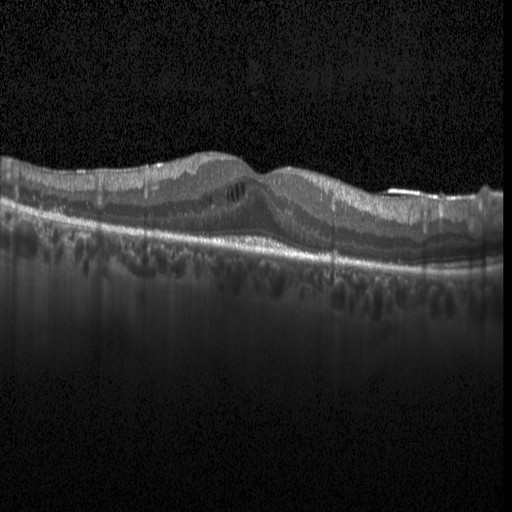
Retinal OCT cross-section, spectral-domain optical coherence tomography, horizontal scan through the fovea.
Assessment: diabetic macular edema (DME).